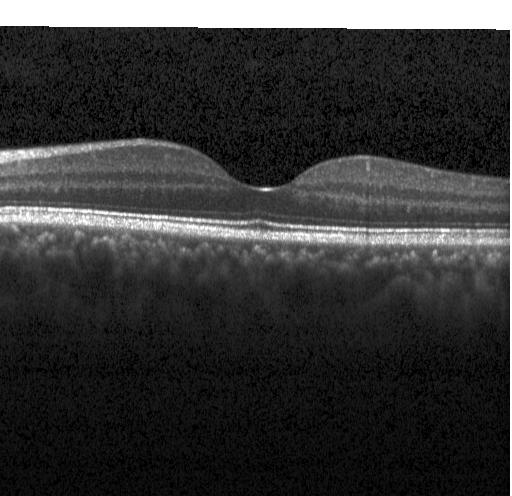
Retinal OCT cross-section.
Neither CNV, DME, nor drusen.